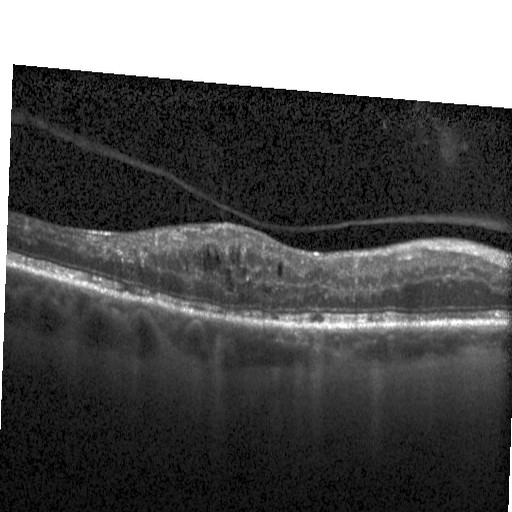

Spectral-domain OCT B-scan: DME.